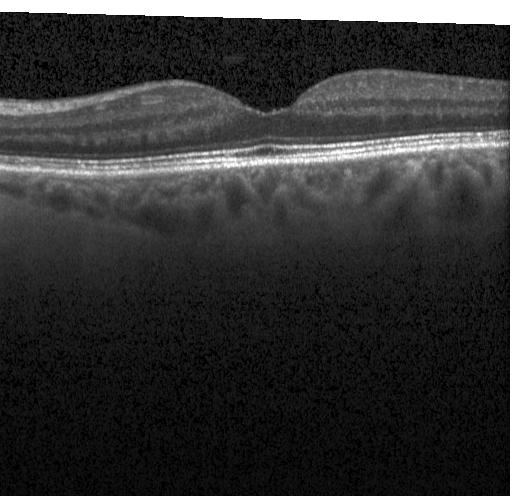 Macular OCT demonstrating neither CNV, DME, nor drusen.